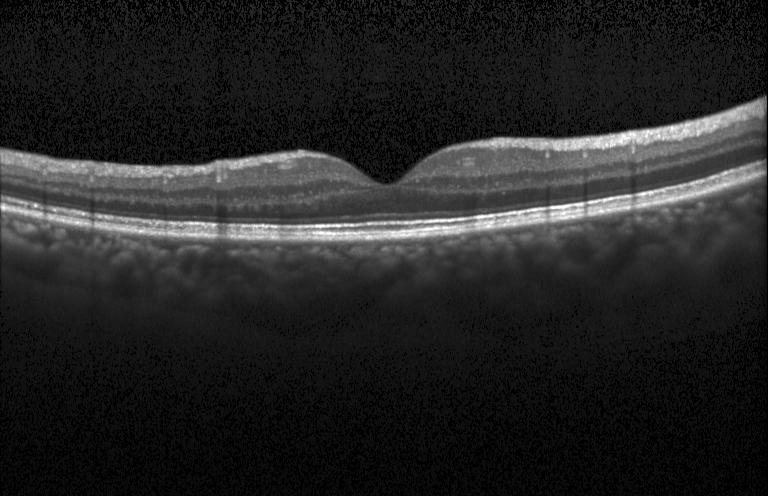 Macular OCT demonstrating neither choroidal neovascularization, diabetic macular edema, nor drusen.